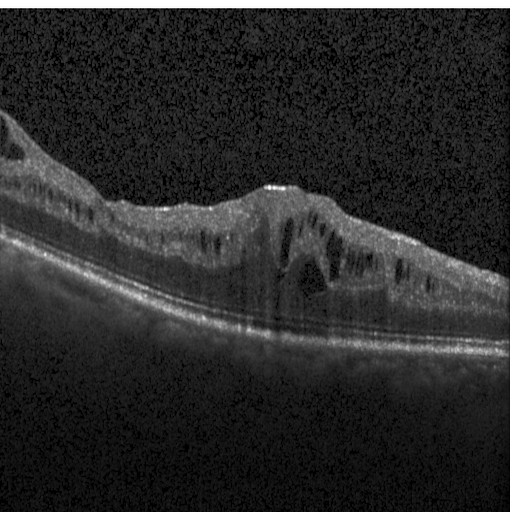 Optical coherence tomography scan
Finding: DME.